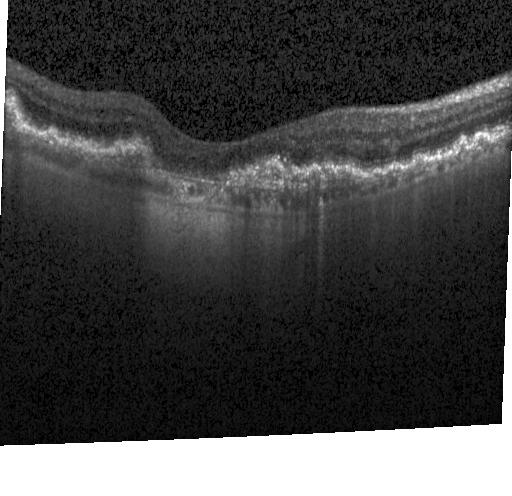

Optical coherence tomography B-scan — This B-scan demonstrates choroidal neovascularization (CNV).